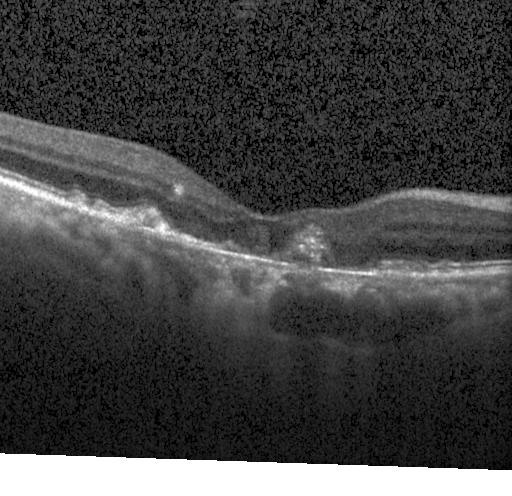

Through the macula. OCT B-scan. Heidelberg Spectralis OCT system. A choroidal neovascular membrane.